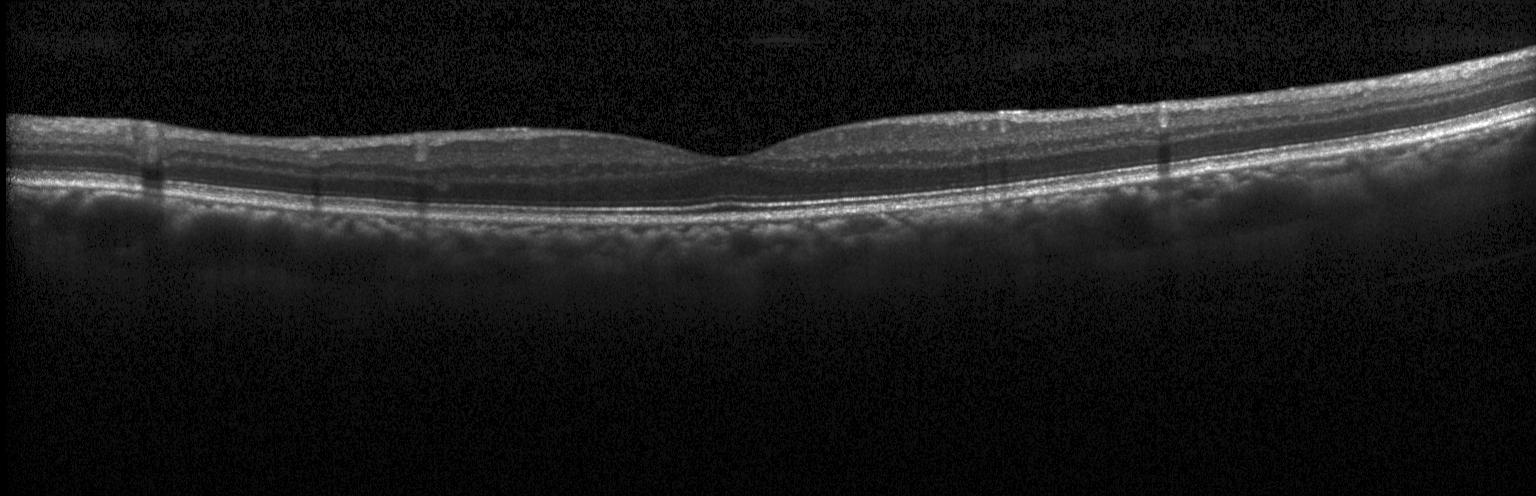

Macular OCT demonstrating no evidence of choroidal neovascularization, diabetic macular edema, or drusen.